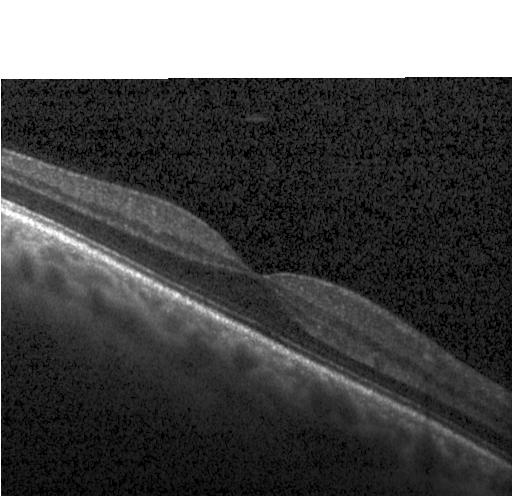
OCT scan showing no evidence of choroidal neovascularization, diabetic macular edema, or drusen.